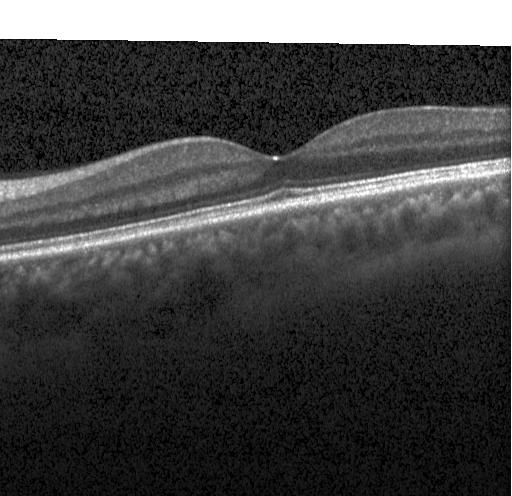 Through the macula. OCT B-scan. Finding: neither choroidal neovascularization, diabetic macular edema, nor drusen.